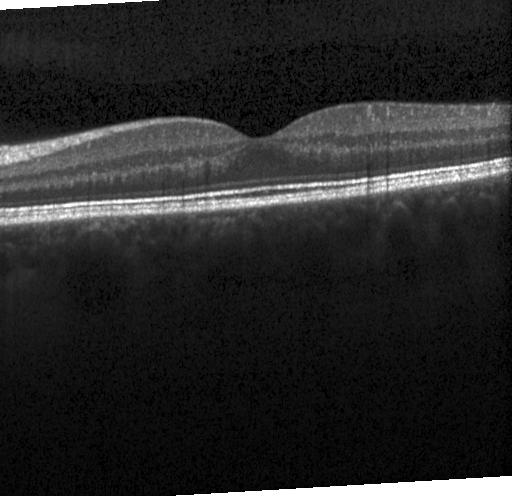
Retinal OCT B-scan
No evidence of choroidal neovascularization, diabetic macular edema, or drusen.